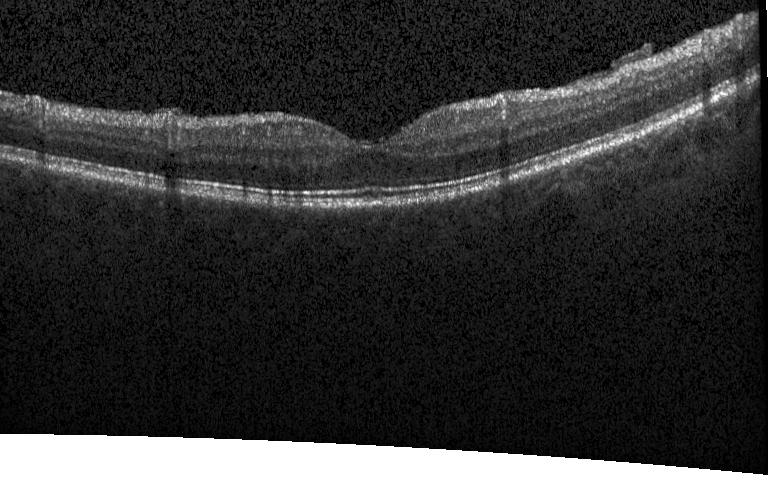

Retinal OCT B-scan, spectral-domain optical coherence tomography, horizontal scan through the fovea, Heidelberg Spectralis OCT system — Macular OCT: neither choroidal neovascularization, diabetic macular edema, nor drusen.